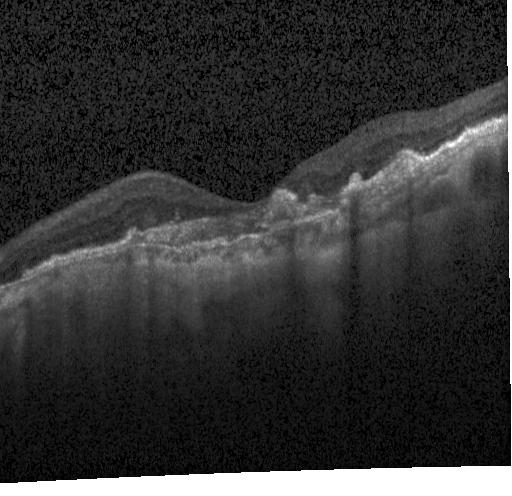 OCT scan showing a choroidal neovascular membrane.